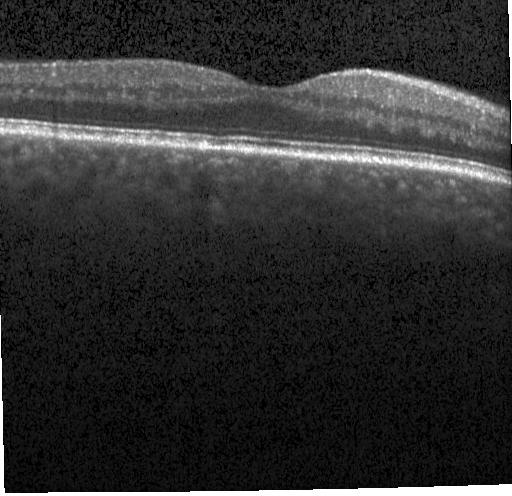

Horizontal scan through the fovea, optical coherence tomography B-scan — No choroidal neovascularization, diabetic macular edema, or drusen.